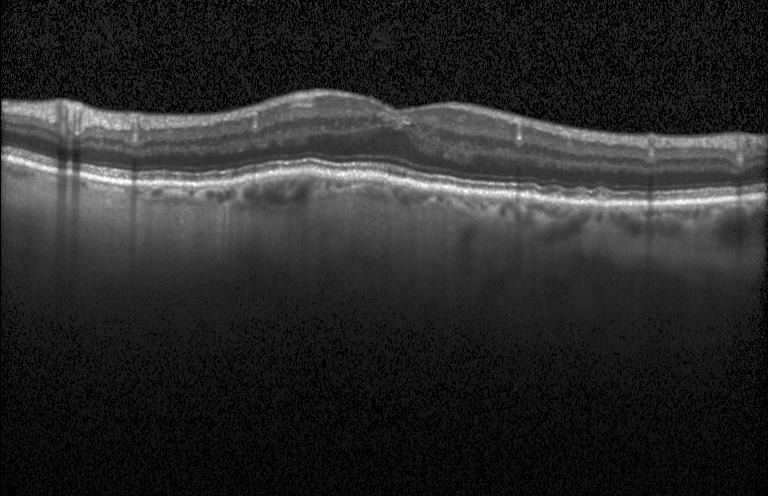
Assessment: multiple drusen.